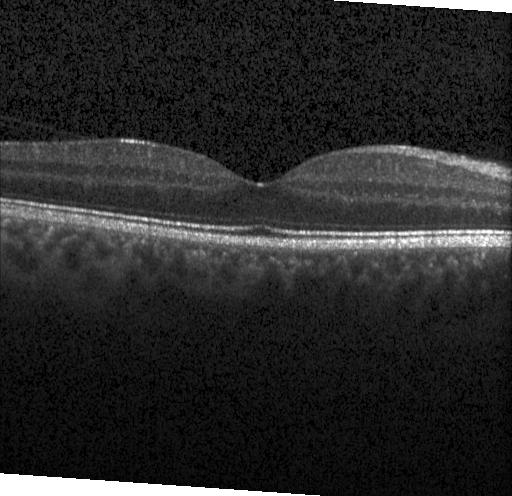 Horizontal scan through the fovea · optical coherence tomography B-scan · acquired on a Heidelberg Spectralis. No CNV, DME, or drusen.